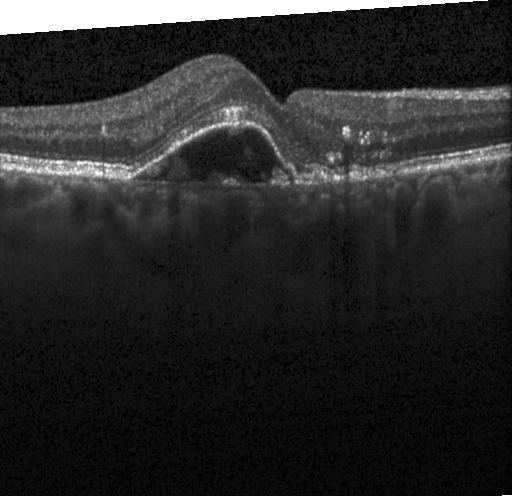
Macular scan · optical coherence tomography scan.
Diagnosis: CNV.